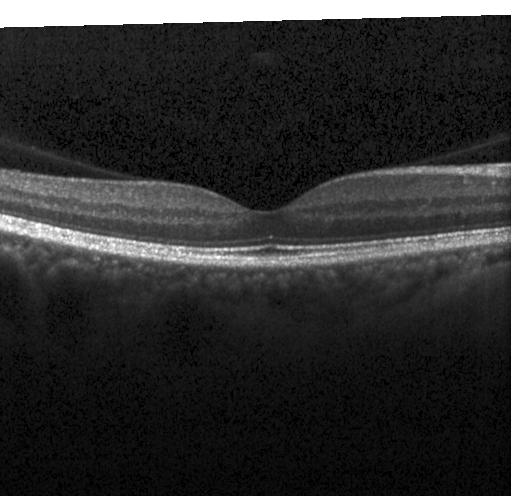
Optical coherence tomography scan
Dx: no CNV, no DME, and no drusen.